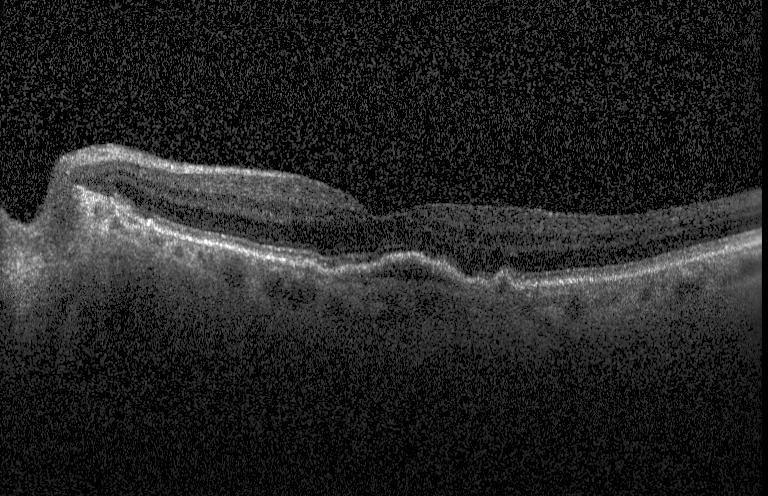 OCT B-scan; spectral-domain OCT; fovea-centered; Heidelberg Spectralis OCT system. Dx: CNV.